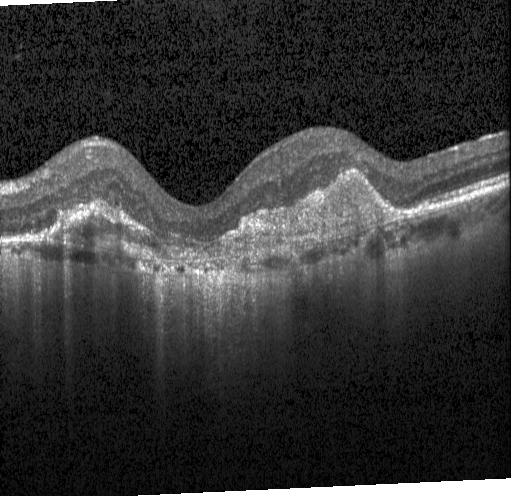
Optical coherence tomography B-scan, acquired on a Heidelberg Spectralis — This B-scan demonstrates choroidal neovascularization (CNV).